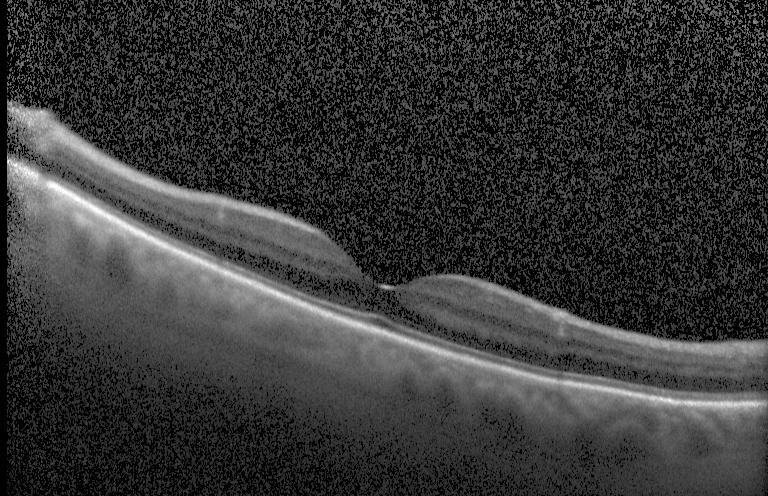
SD-OCT, retinal OCT cross-section.
Impression: no evidence of choroidal neovascularization, diabetic macular edema, or drusen.